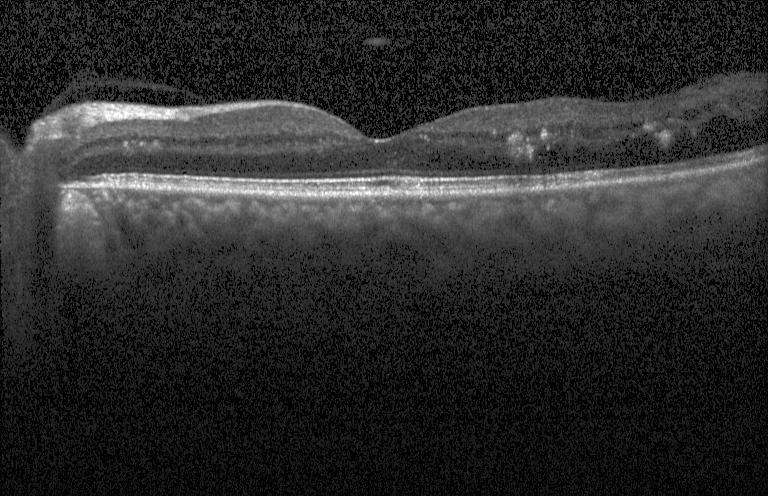

Macular OCT demonstrating diabetic macular edema (DME).